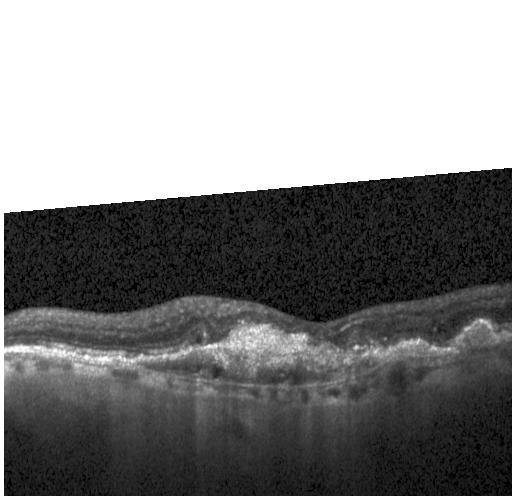
OCT B-scan. Finding: a choroidal neovascular membrane.